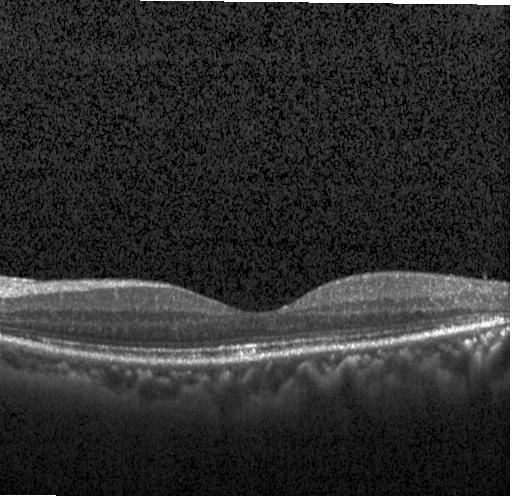

Spectral-domain optical coherence tomography, OCT B-scan, centered on the fovea, Heidelberg Spectralis OCT system. Assessment: no evidence of CNV, DME, or drusen.